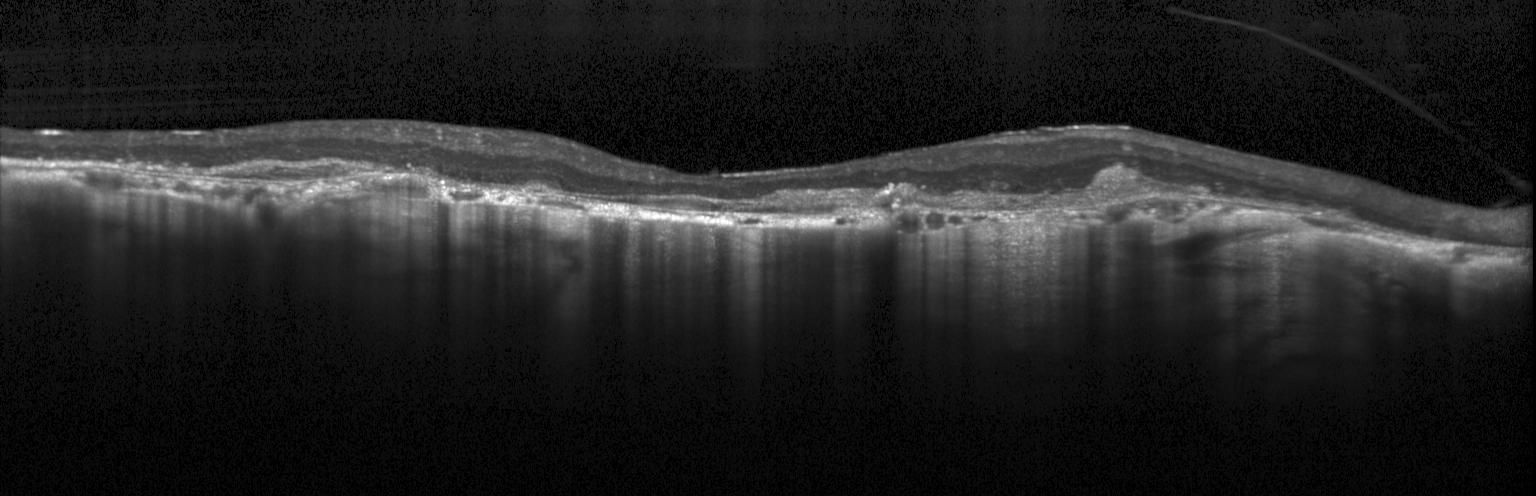

Spectral-domain OCT B-scan: CNV.